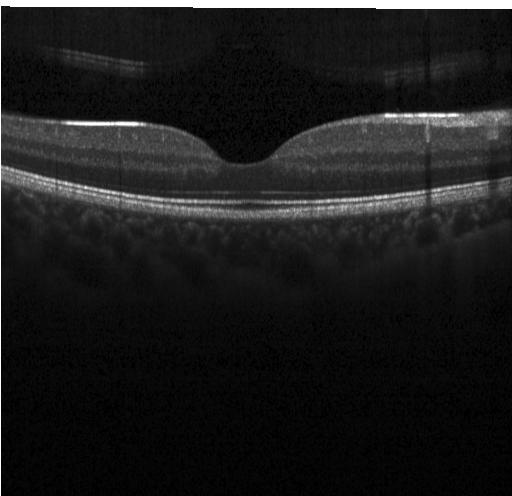
Spectral-domain OCT. OCT B-scan. Centered on the fovea
Diagnosis: neither choroidal neovascularization, diabetic macular edema, nor drusen.